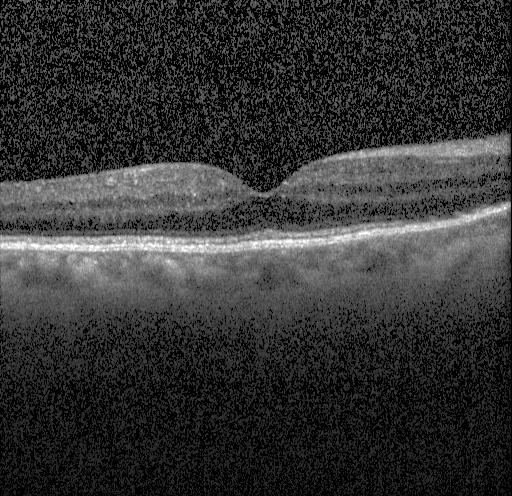

Spectral-domain optical coherence tomography; optical coherence tomography scan; macular scan; acquired on a Heidelberg Spectralis.
Macular OCT: neither CNV, DME, nor drusen.